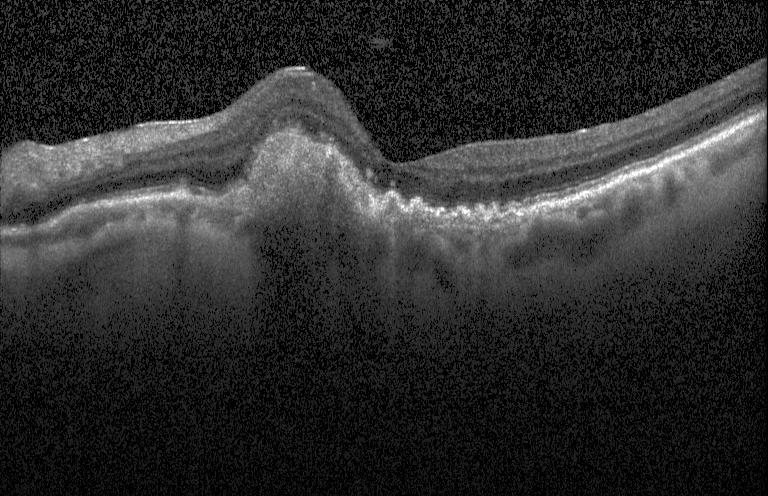
Dx: a choroidal neovascular membrane.